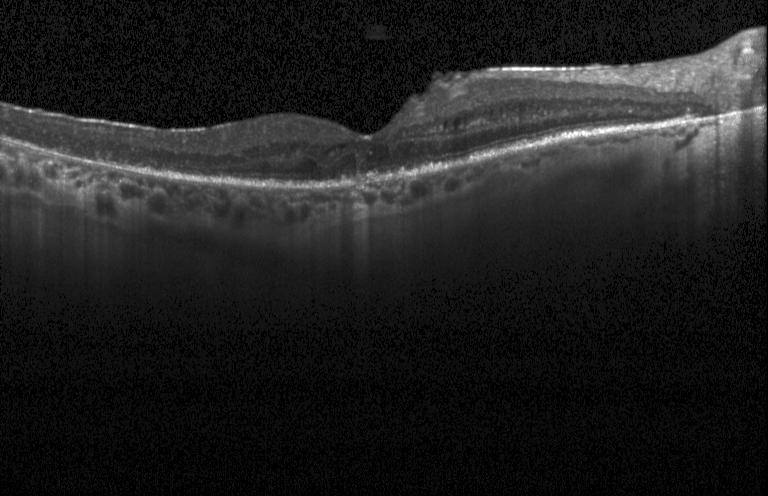 Spectral-domain optical coherence tomography; Heidelberg Spectralis; OCT line scan; macular scan — Macular OCT: no CNV, DME, or drusen.